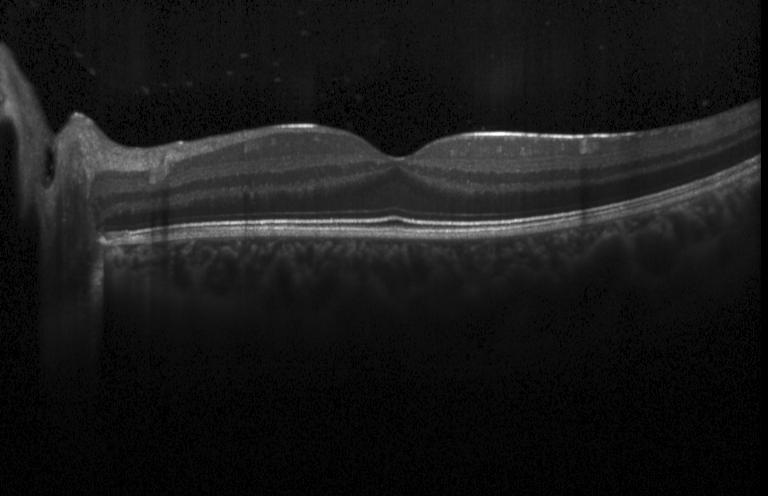

Assessment: no choroidal neovascularization, no diabetic macular edema, and no drusen.